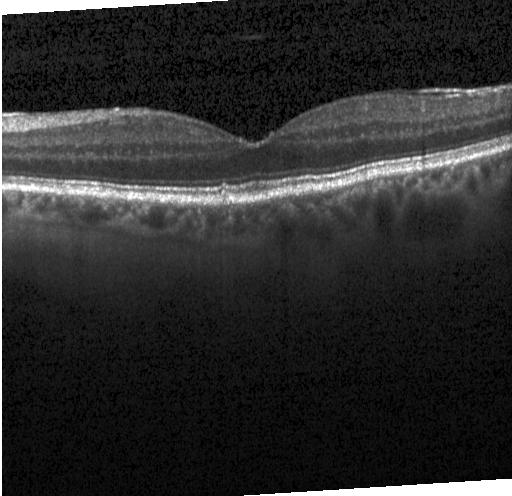 OCT line scan. Heidelberg Spectralis OCT system. Horizontal scan through the fovea. Assessment: multiple drusen.